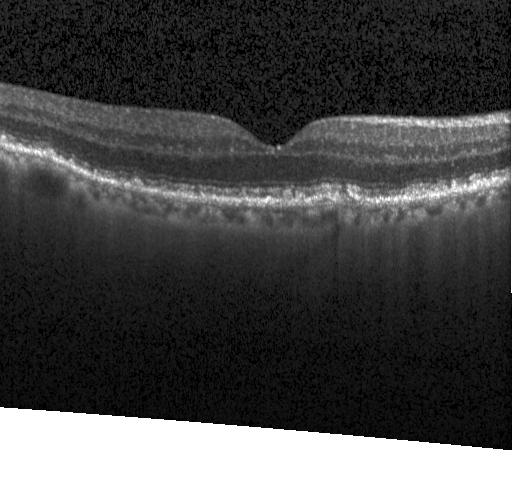

OCT B-scan showing sub-RPE drusenoid deposits.